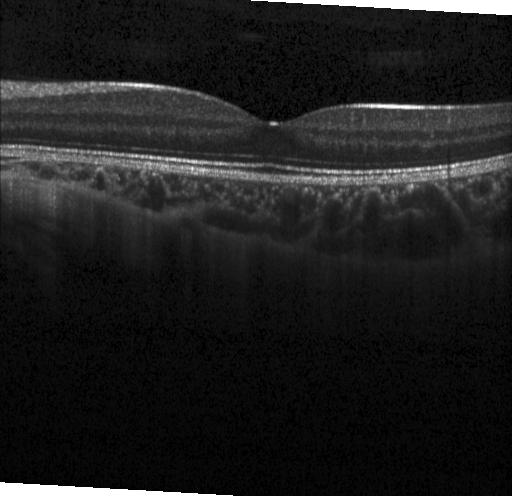 Fovea-centered, spectral-domain optical coherence tomography, Heidelberg Spectralis, retinal OCT B-scan
Macular OCT: no CNV, DME, or drusen.